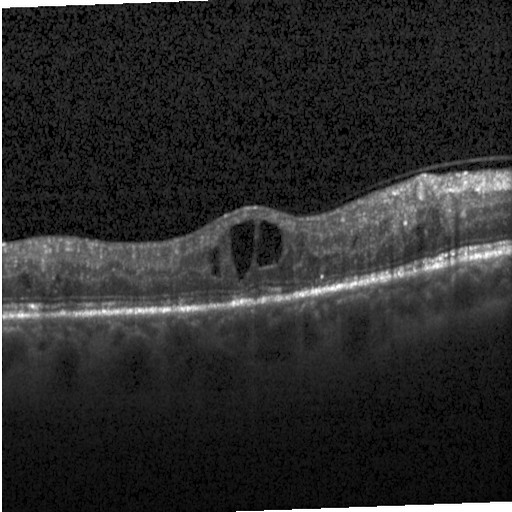
OCT B-scan showing diabetic macular edema.